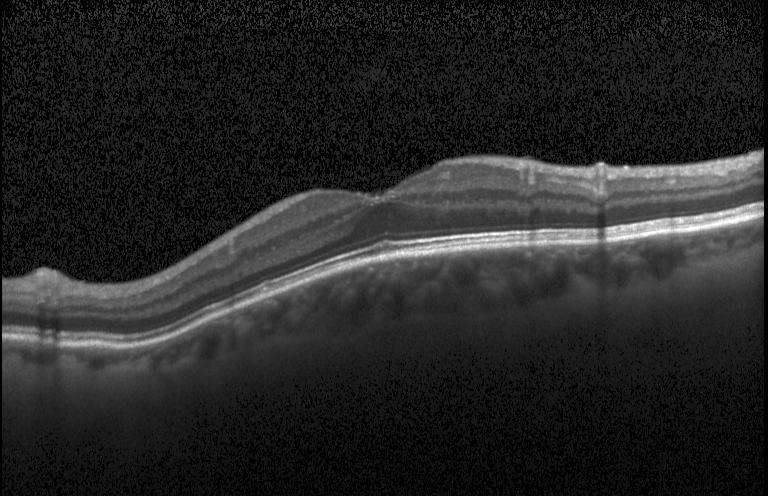

Assessment: no evidence of choroidal neovascularization, diabetic macular edema, or drusen.